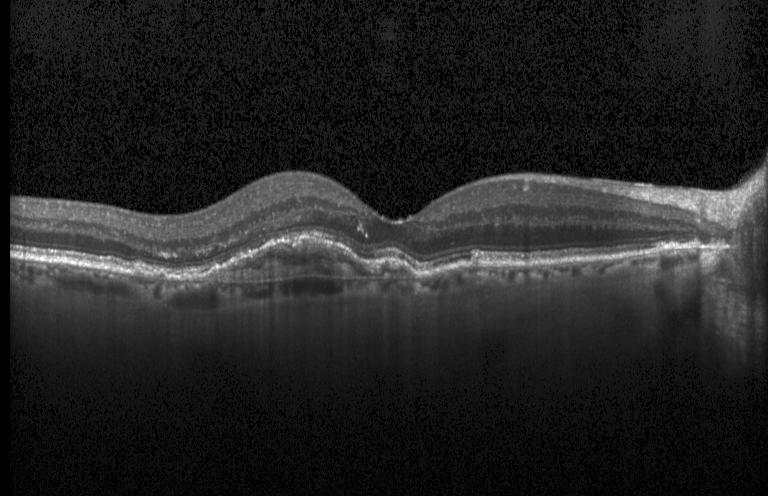
This B-scan demonstrates choroidal neovascularization (CNV).